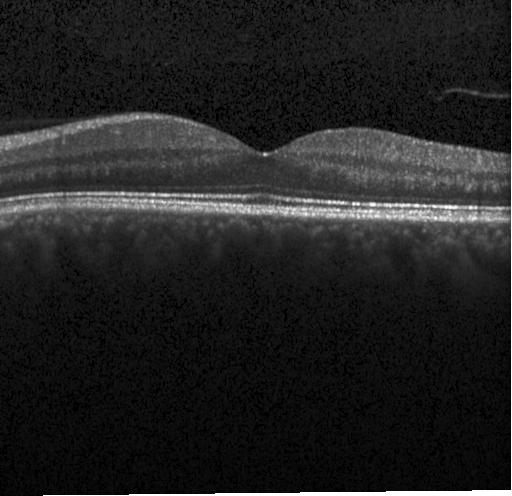
Macular OCT demonstrating no choroidal neovascularization, diabetic macular edema, or drusen.